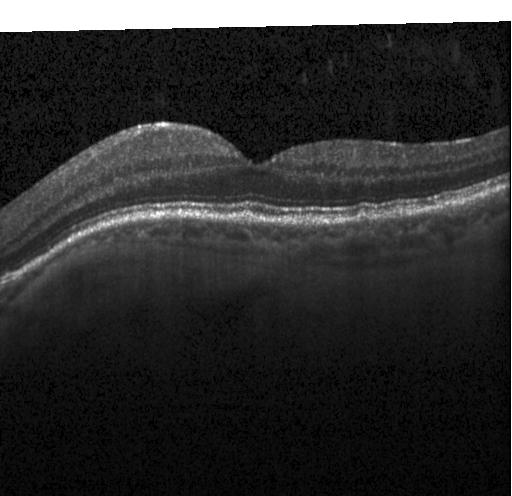

Assessment: sub-RPE drusenoid deposits.